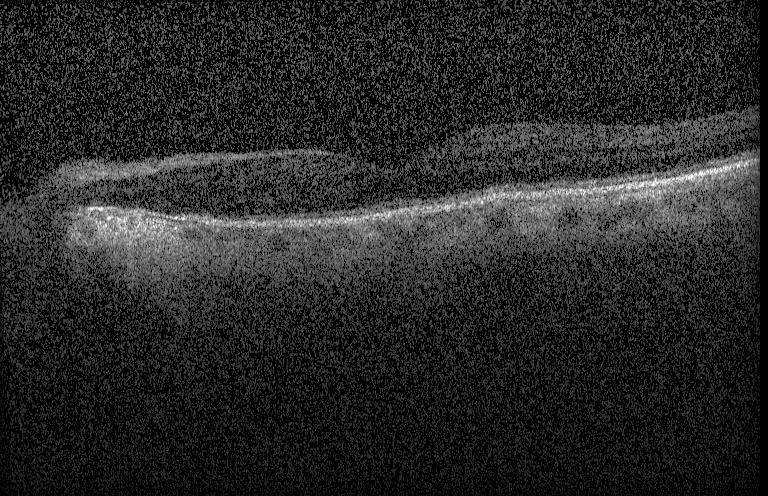

OCT B-scan. Macular OCT: no CNV, no DME, and no drusen.